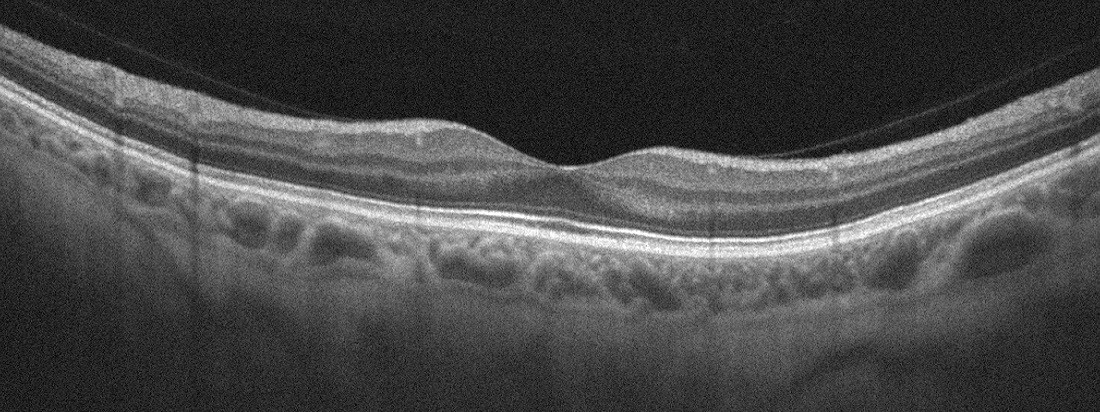
OCT line scan, fovea-centered, Optovue Avanti RTVue XR.
Impression: no evidence of AMD, DME, ERM, RAO, RVO, or VID.